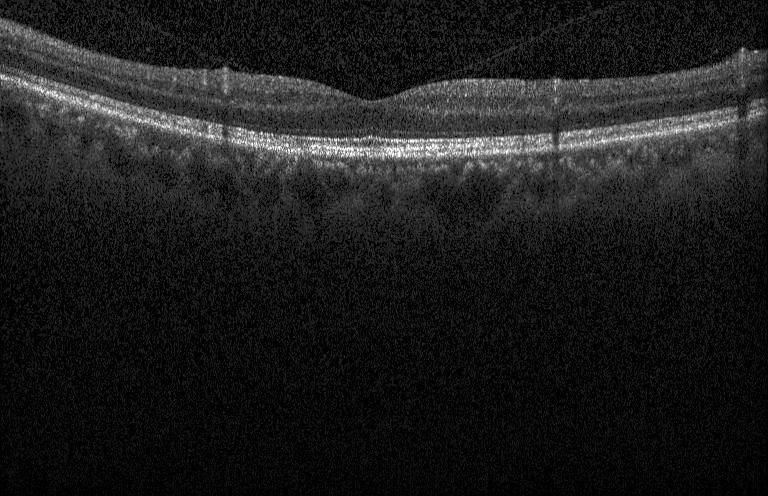

Optical coherence tomography B-scan. Diagnosis: no CNV, DME, or drusen.